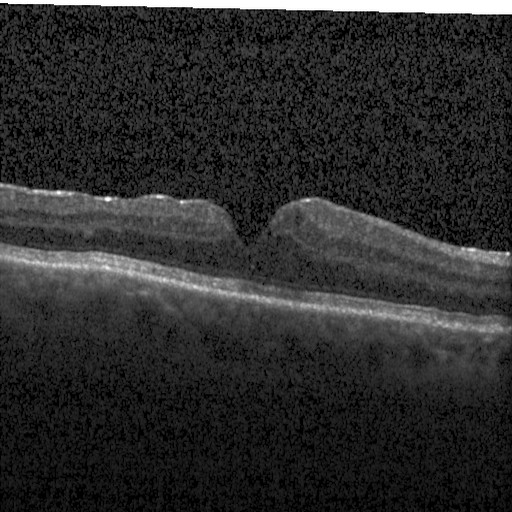 DME.